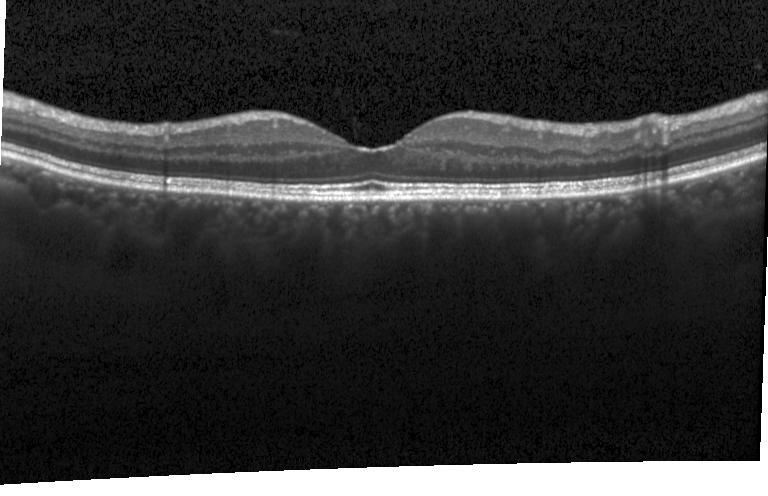

Retinal OCT cross-section, instrument: Heidelberg Spectralis. Dx: no evidence of choroidal neovascularization, diabetic macular edema, or drusen.